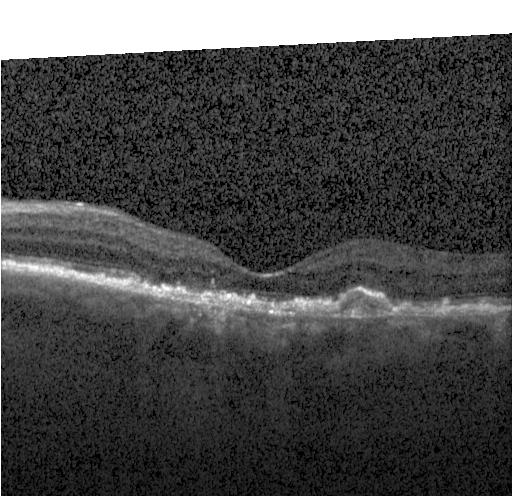

Heidelberg Spectralis OCT system · horizontal scan through the fovea · optical coherence tomography B-scan.
This B-scan demonstrates a choroidal neovascular membrane.